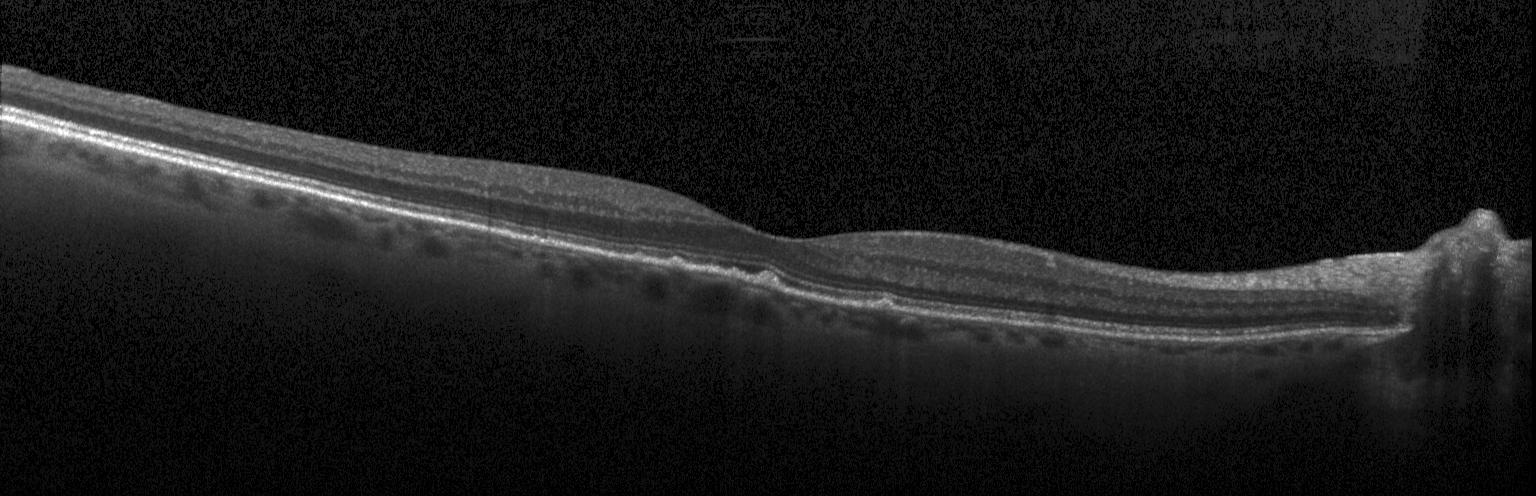

Retinal OCT cross-section. Spectral-domain OCT. Acquired on a Heidelberg Spectralis. Through the macula — Impression: multiple drusen.